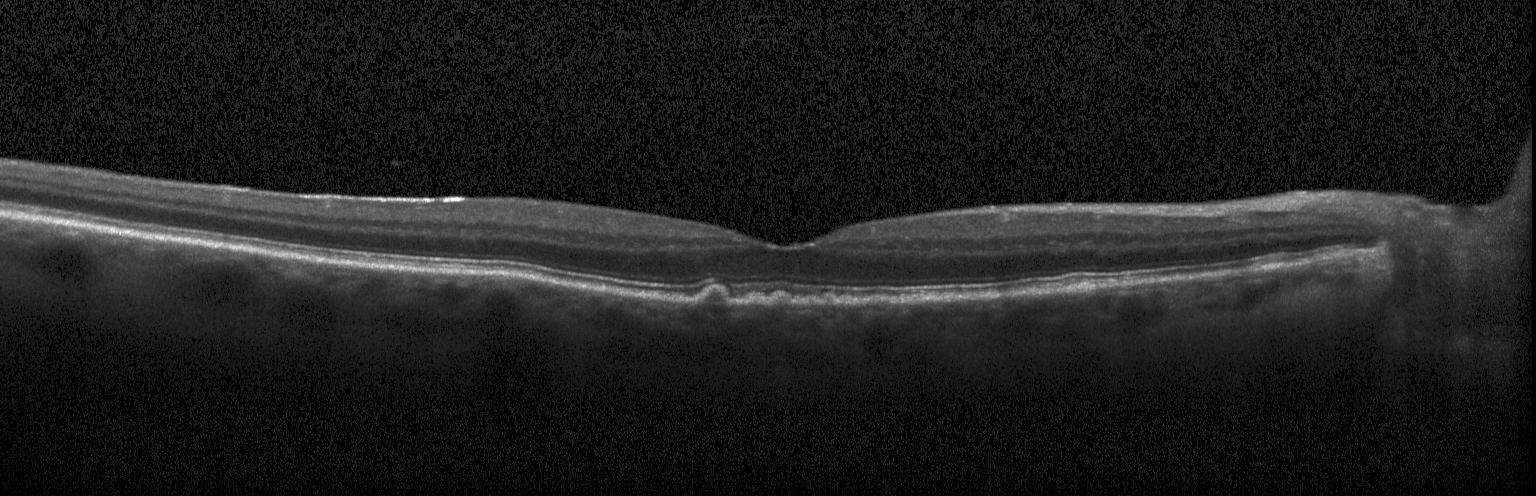
Acquired on a Heidelberg Spectralis; OCT line scan.
The scan shows drusen.